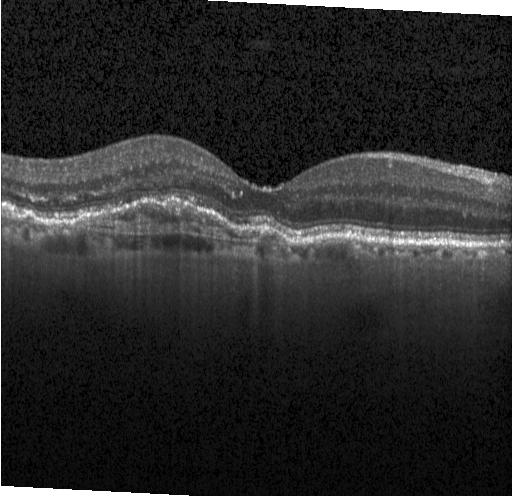

Optical coherence tomography scan, spectral-domain optical coherence tomography, acquired on a Heidelberg Spectralis, macular scan
Macular OCT: a choroidal neovascular membrane.